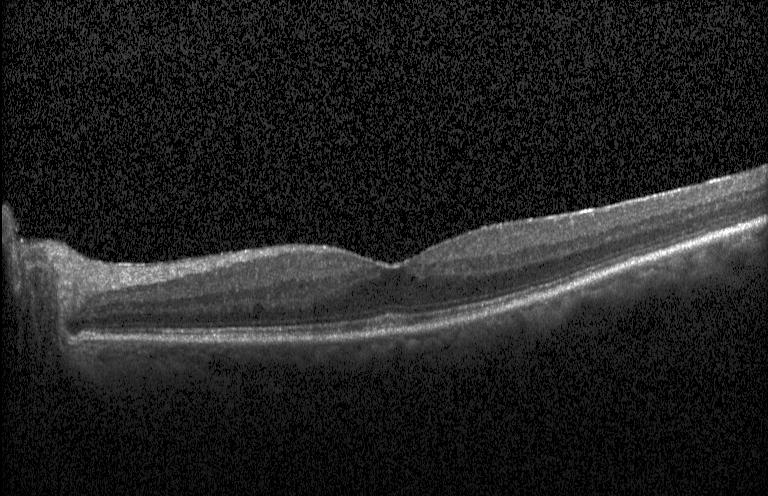

Impression: DME.